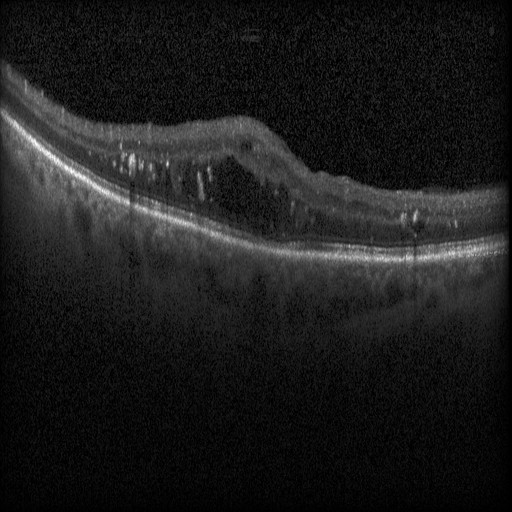

Retinal OCT cross-section; SD-OCT
Diabetic macular edema (DME).